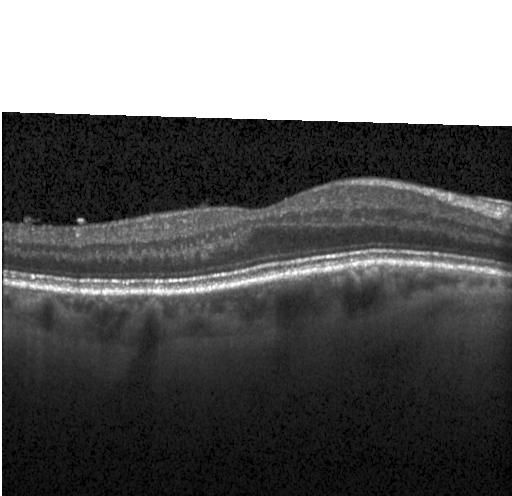
Heidelberg Spectralis OCT system · horizontal scan through the fovea · OCT line scan — The scan shows neither CNV, DME, nor drusen.